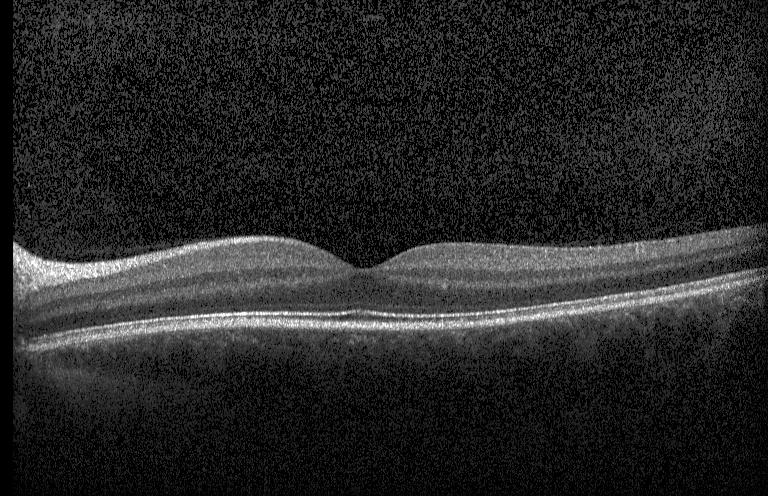

Assessment: neither choroidal neovascularization, diabetic macular edema, nor drusen.